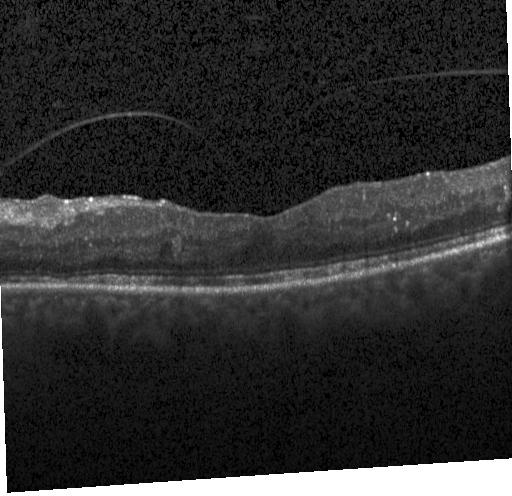
Dx: diabetic macular edema (DME).